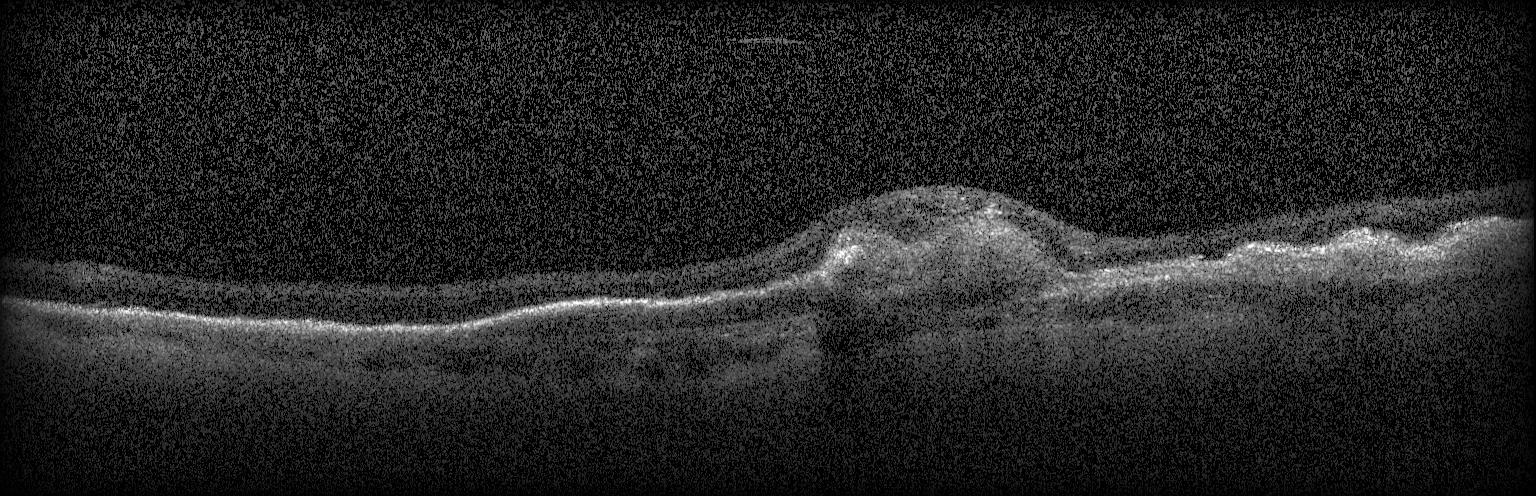
Acquired on a Heidelberg Spectralis; optical coherence tomography B-scan.
Diagnosis: choroidal neovascularization.